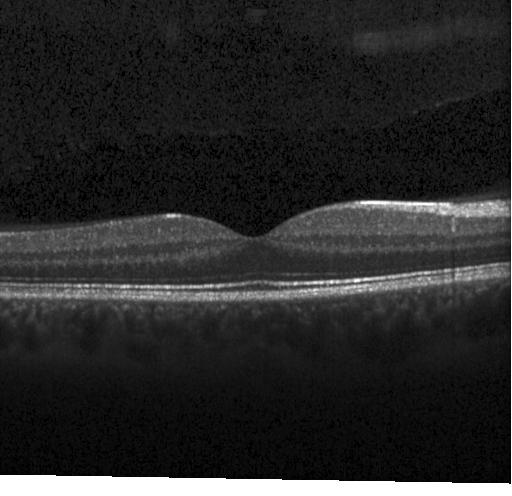 No choroidal neovascularization, diabetic macular edema, or drusen.